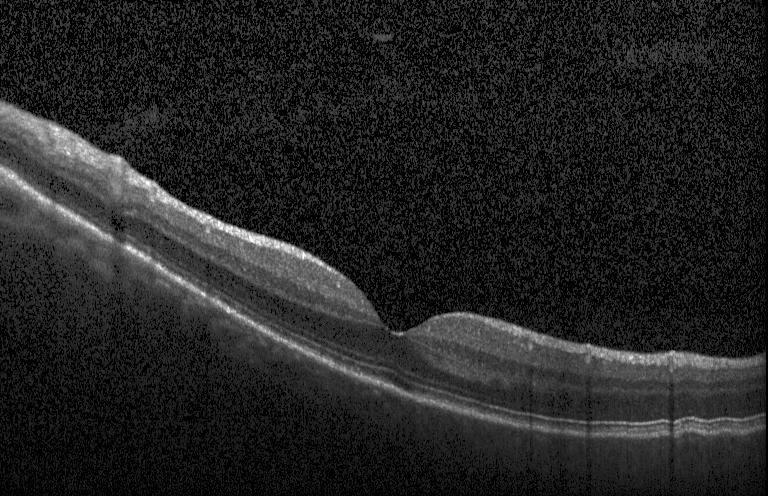
Retinal OCT B-scan · Heidelberg Spectralis OCT system · fovea-centered.
No evidence of choroidal neovascularization, diabetic macular edema, or drusen.